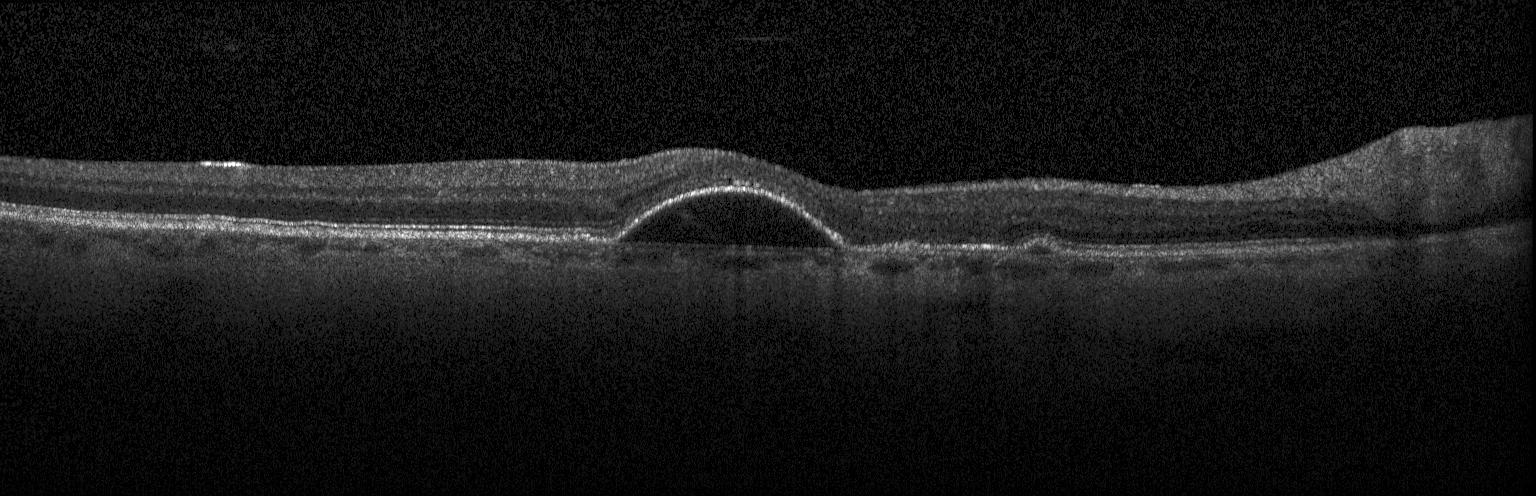

This B-scan demonstrates a choroidal neovascular membrane.